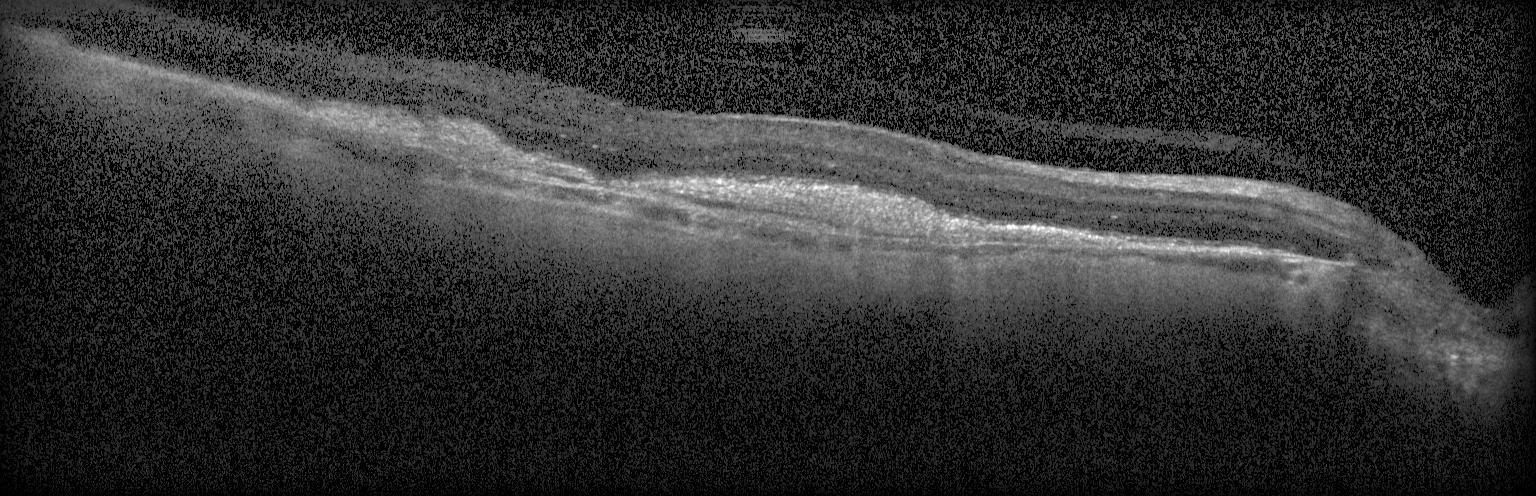 The scan shows choroidal neovascularization.